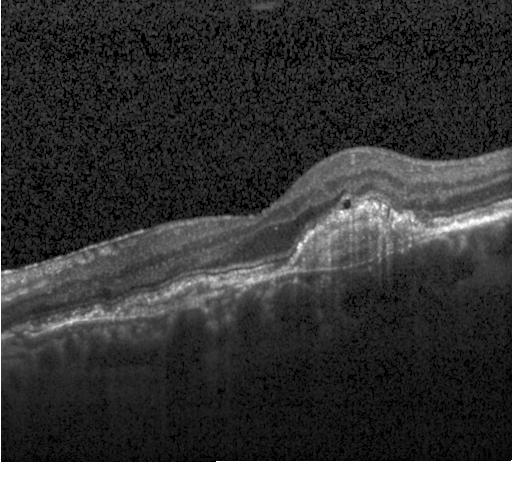
Assessment: CNV.